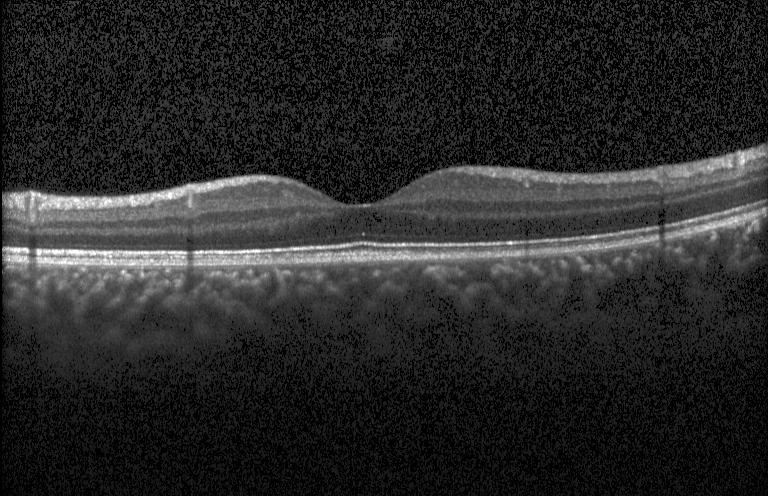
OCT scan showing neither choroidal neovascularization, diabetic macular edema, nor drusen.